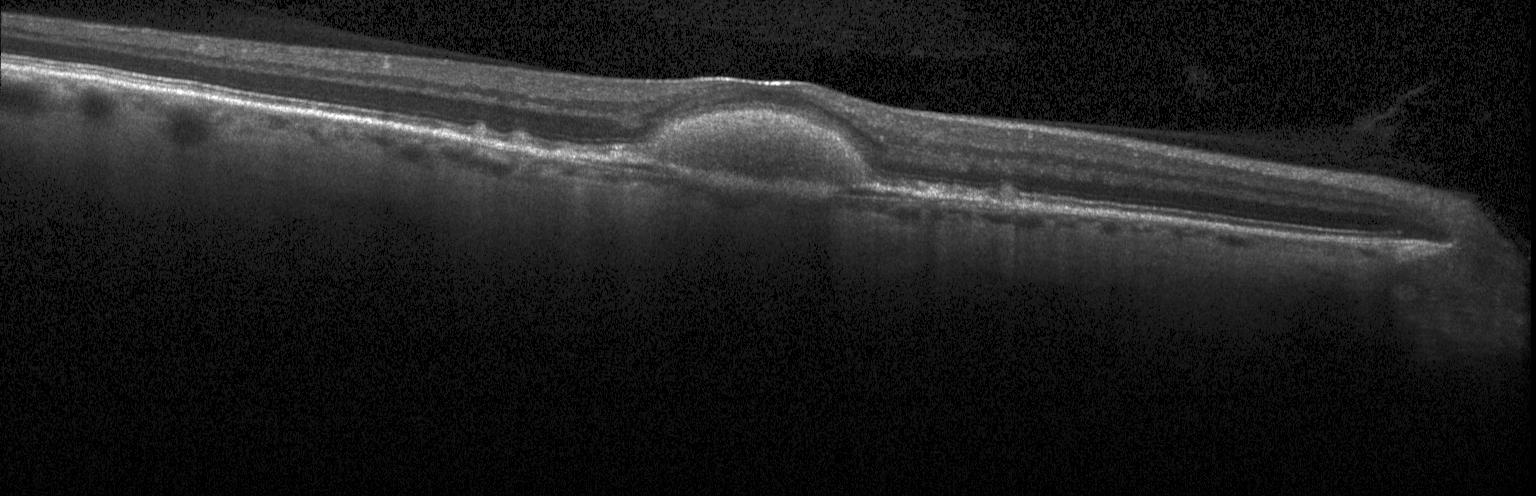

Instrument: Heidelberg Spectralis · centered on the fovea · optical coherence tomography scan · spectral-domain OCT.
Finding: choroidal neovascularization (CNV).